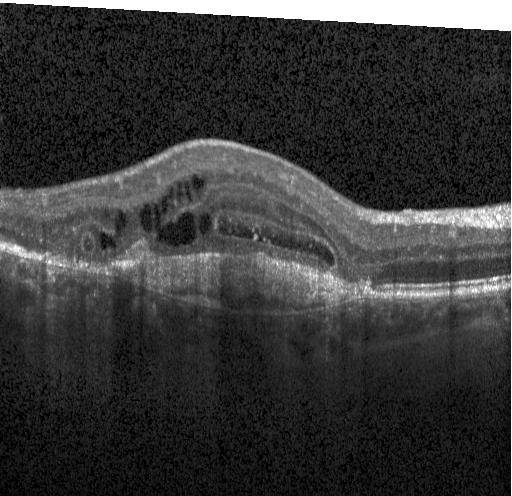 Assessment: a choroidal neovascular membrane.